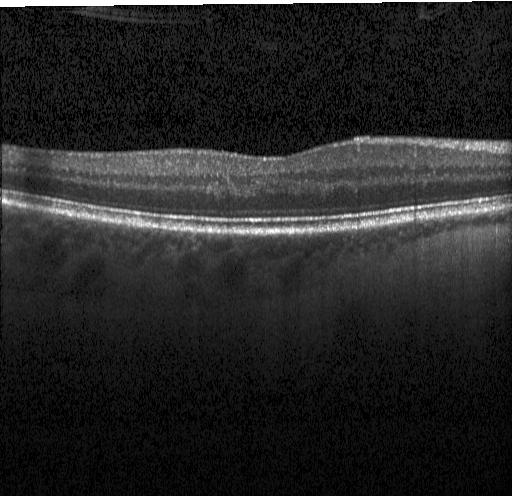 OCT B-scan
OCT finding: no evidence of choroidal neovascularization, diabetic macular edema, or drusen.